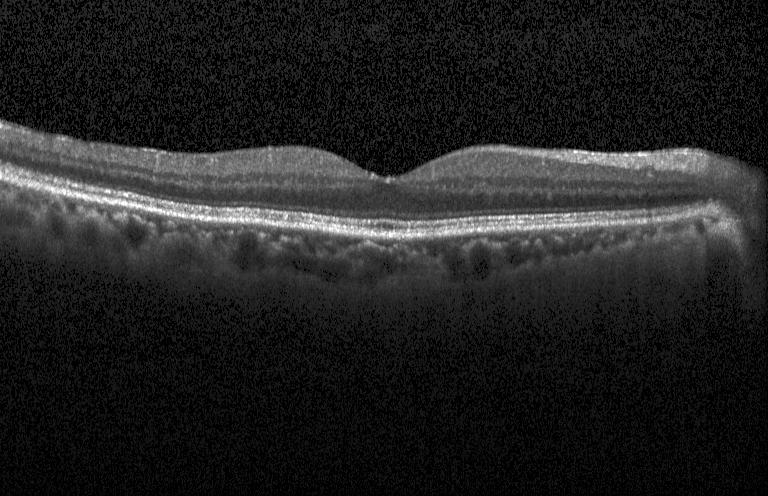 Horizontal scan through the fovea; retinal OCT B-scan; spectral-domain OCT; Heidelberg Spectralis OCT system.
Finding: neither choroidal neovascularization, diabetic macular edema, nor drusen.